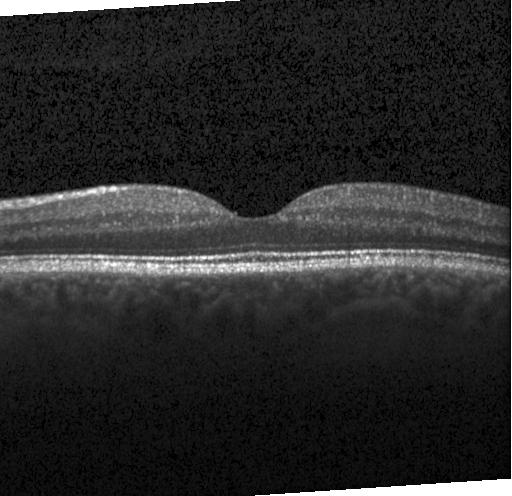 Impression: no evidence of choroidal neovascularization, diabetic macular edema, or drusen.